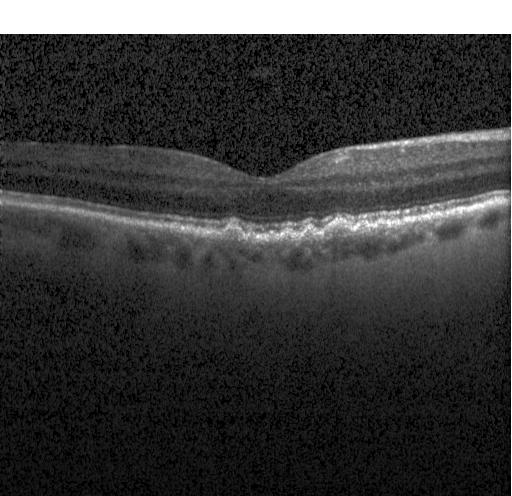 Centered on the fovea · OCT line scan · SD-OCT
Diagnosis: sub-RPE drusenoid deposits.